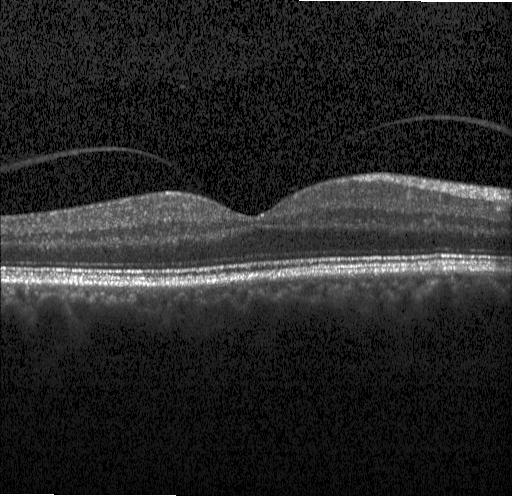
Macular OCT: no evidence of choroidal neovascularization, diabetic macular edema, or drusen.